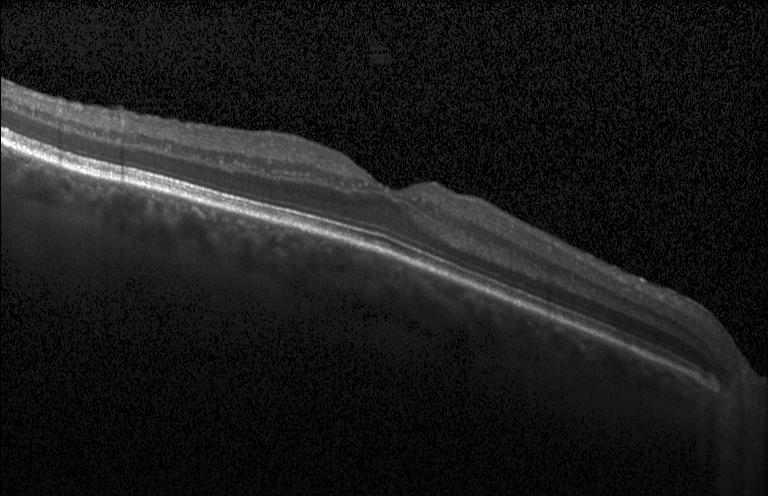 Finding: neither choroidal neovascularization, diabetic macular edema, nor drusen.